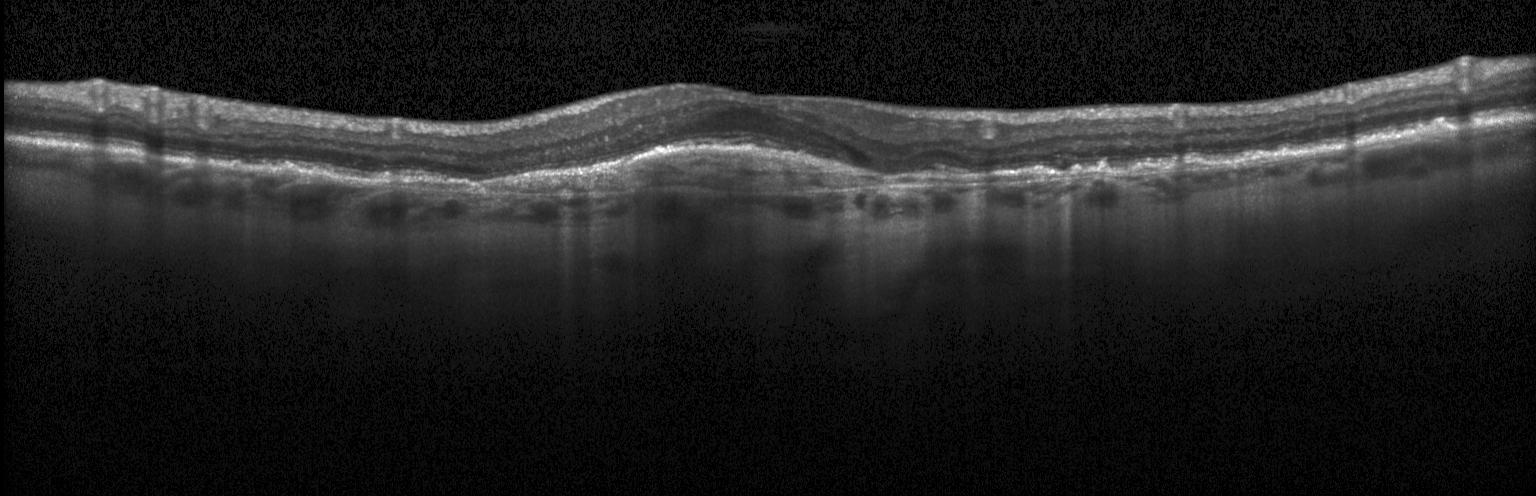

OCT B-scan; instrument: Heidelberg Spectralis.
Diagnosis: choroidal neovascularization.